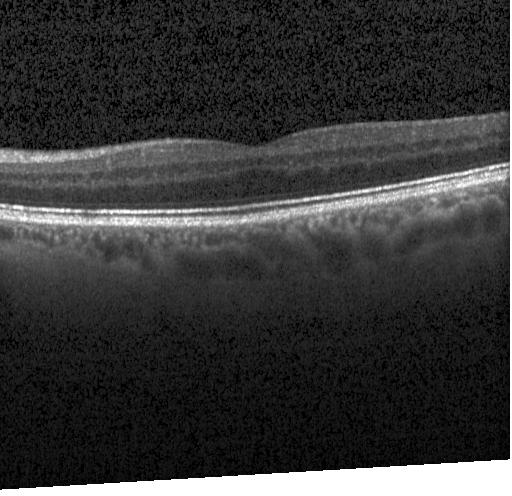

Optical coherence tomography B-scan · spectral-domain optical coherence tomography · Heidelberg Spectralis
Neither choroidal neovascularization, diabetic macular edema, nor drusen.